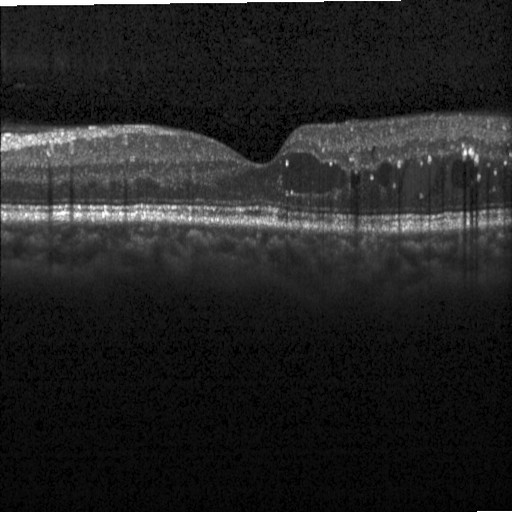

Optical coherence tomography scan, macular scan
Finding: diabetic macular edema.